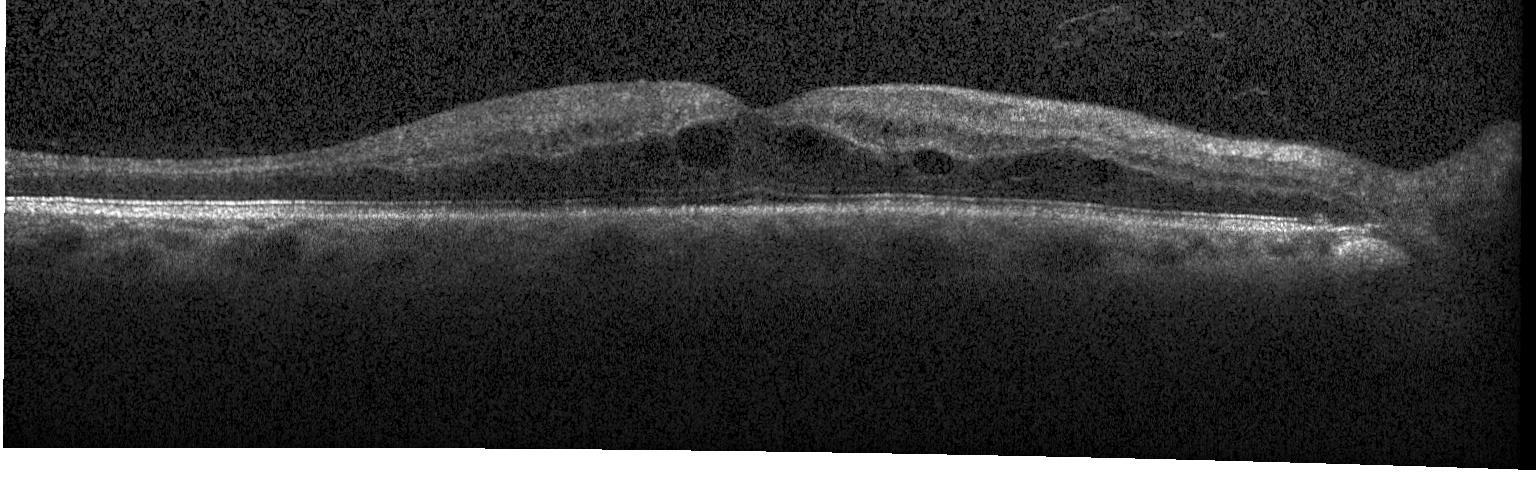
Optical coherence tomography B-scan. Macular scan.
Dx: DME.